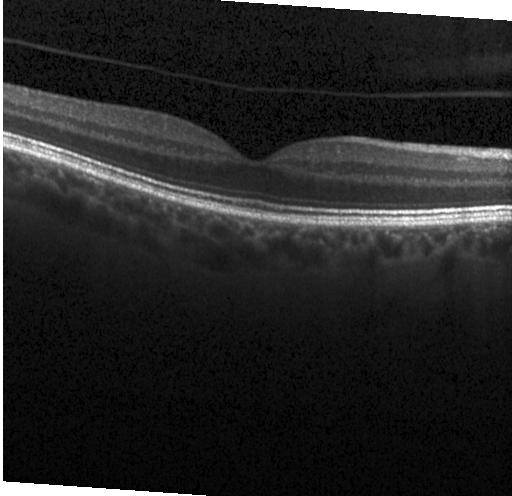

OCT line scan
No evidence of choroidal neovascularization, diabetic macular edema, or drusen.